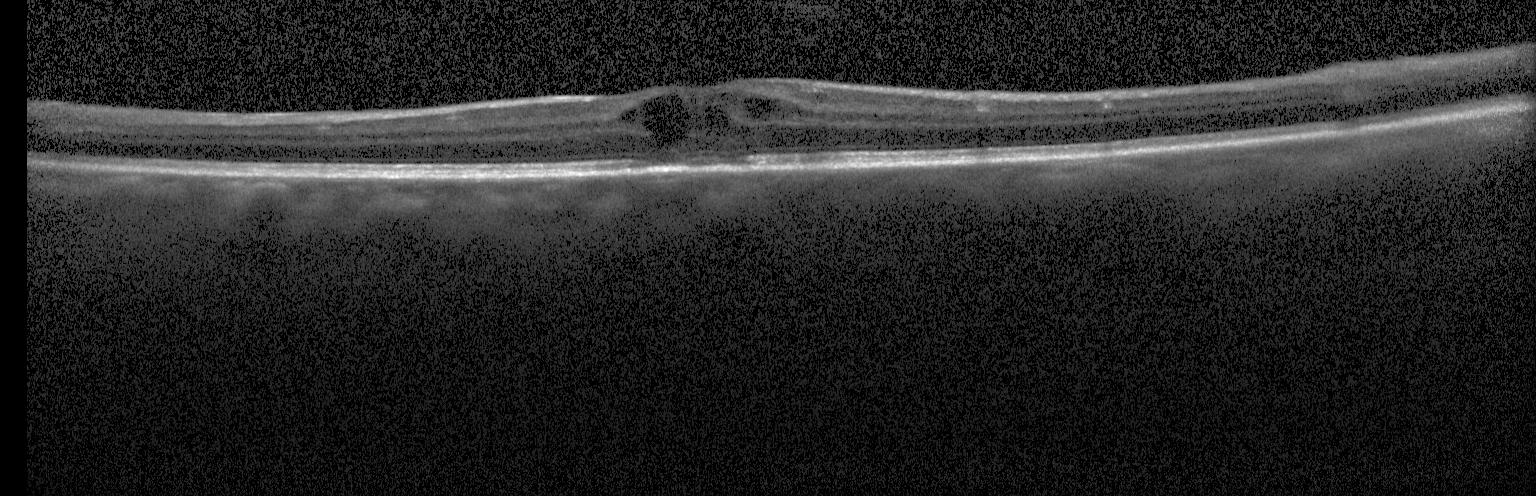

Spectral-domain OCT, acquired on a Heidelberg Spectralis, retinal OCT B-scan, fovea-centered.
OCT finding: diabetic macular edema.